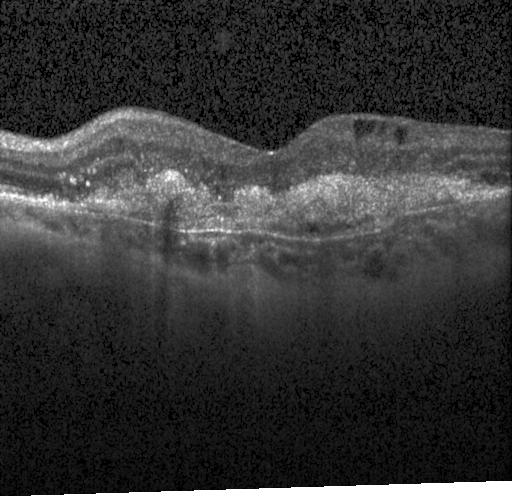
OCT B-scan.
Choroidal neovascularization.